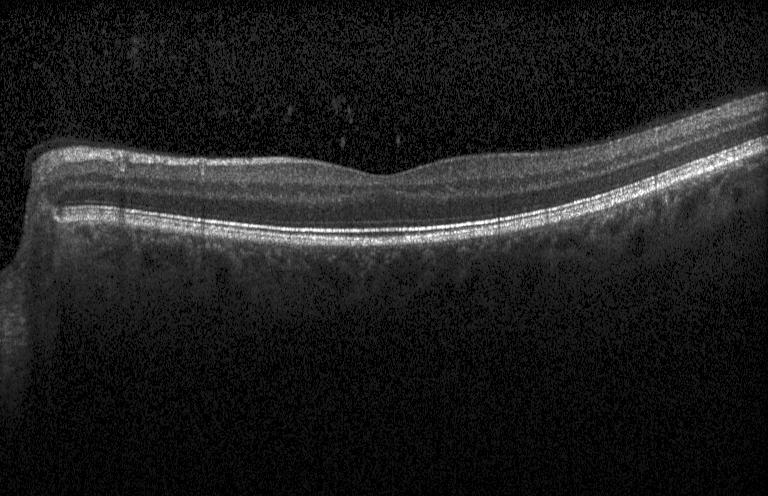
OCT B-scan showing no choroidal neovascularization, no diabetic macular edema, and no drusen.